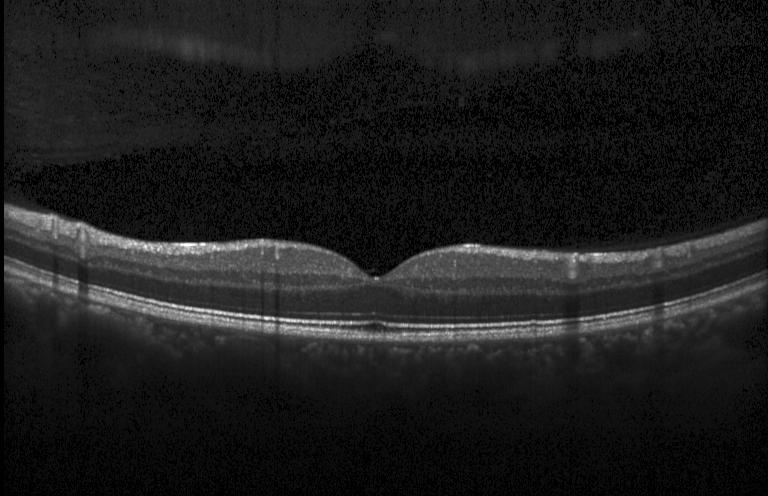

OCT B-scan; spectral-domain OCT. OCT finding: neither choroidal neovascularization, diabetic macular edema, nor drusen.